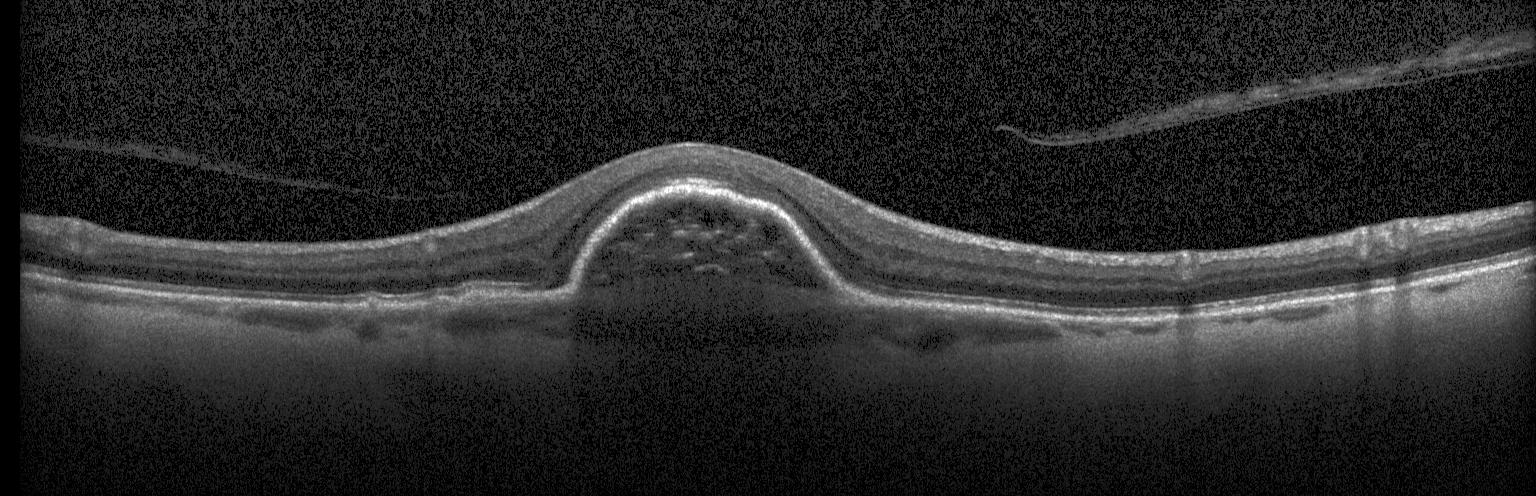
OCT line scan. Spectral-domain optical coherence tomography.
OCT finding: CNV.